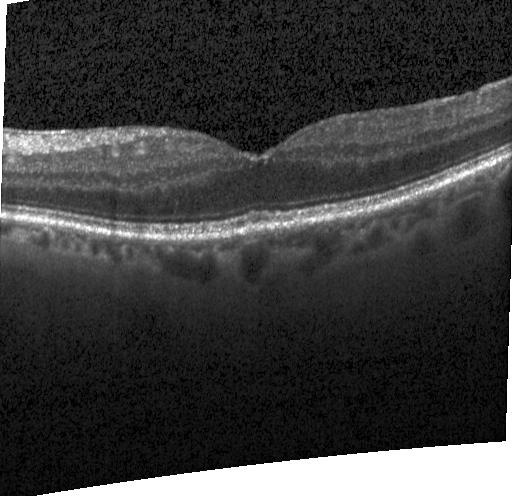

Macular scan · OCT line scan · spectral-domain optical coherence tomography — Diagnosis: no choroidal neovascularization, diabetic macular edema, or drusen.